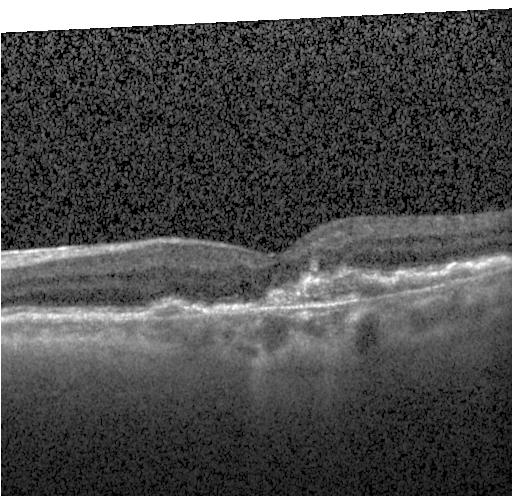 Optical coherence tomography B-scan. Spectral-domain optical coherence tomography
Choroidal neovascularization.